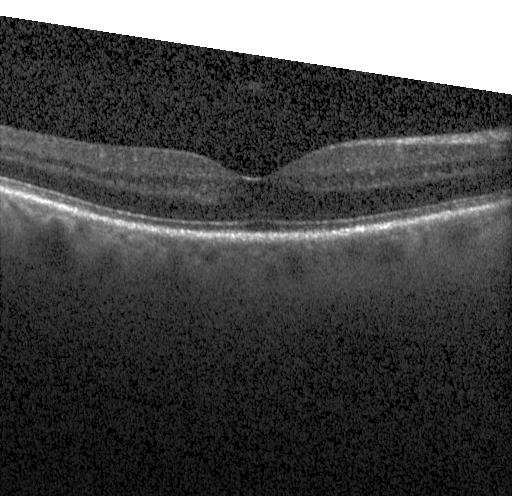
Retinal OCT B-scan. Instrument: Heidelberg Spectralis.
Finding: neither CNV, DME, nor drusen.